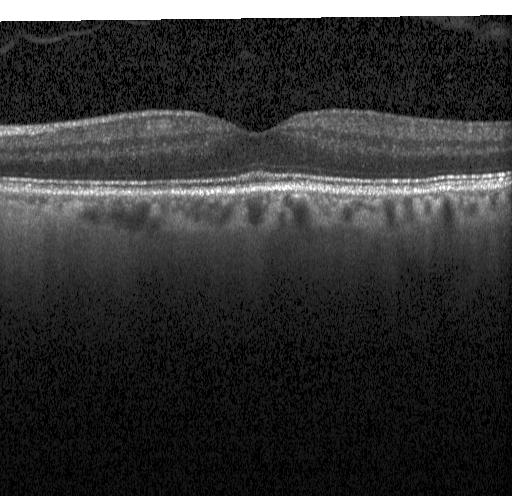

Through the macula, optical coherence tomography scan, spectral-domain OCT
Assessment: no evidence of choroidal neovascularization, diabetic macular edema, or drusen.